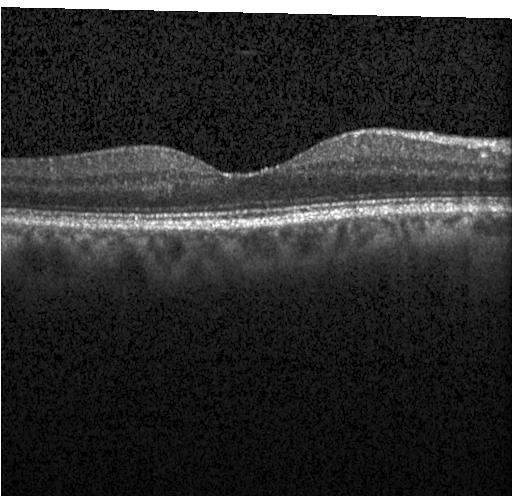

Finding: neither CNV, DME, nor drusen.